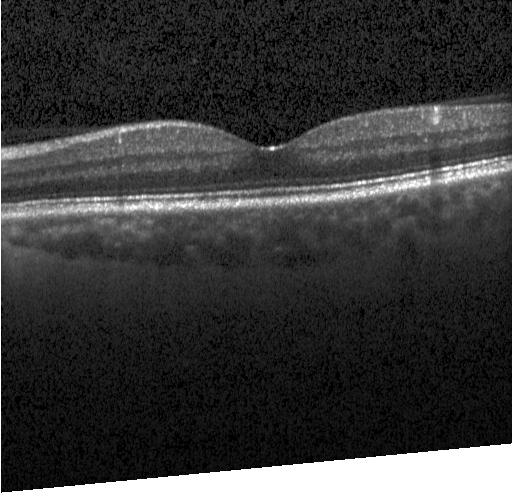

Spectral-domain OCT B-scan: no evidence of choroidal neovascularization, diabetic macular edema, or drusen.